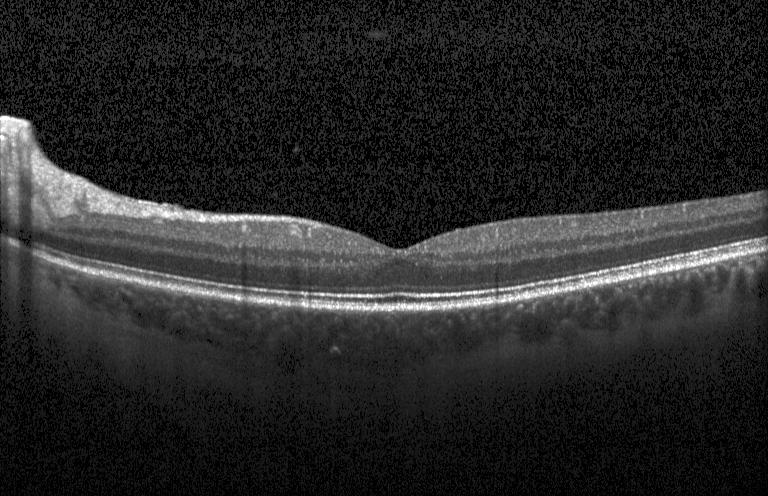
Finding: neither choroidal neovascularization, diabetic macular edema, nor drusen.